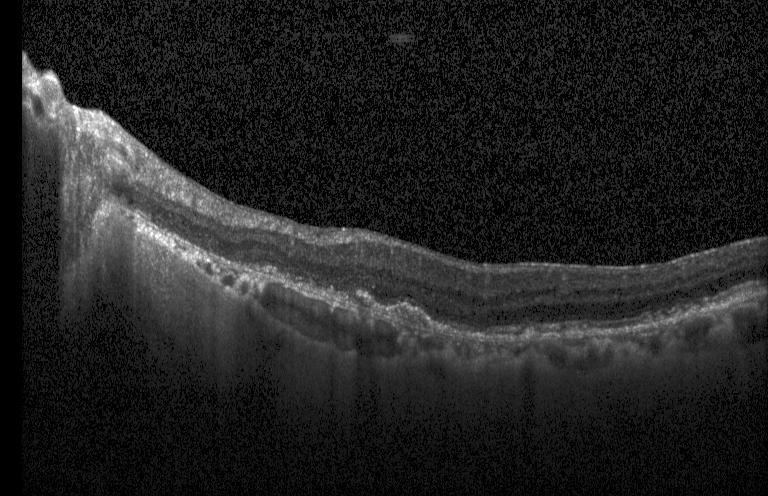

Fovea-centered, optical coherence tomography B-scan. OCT finding: a choroidal neovascular membrane.